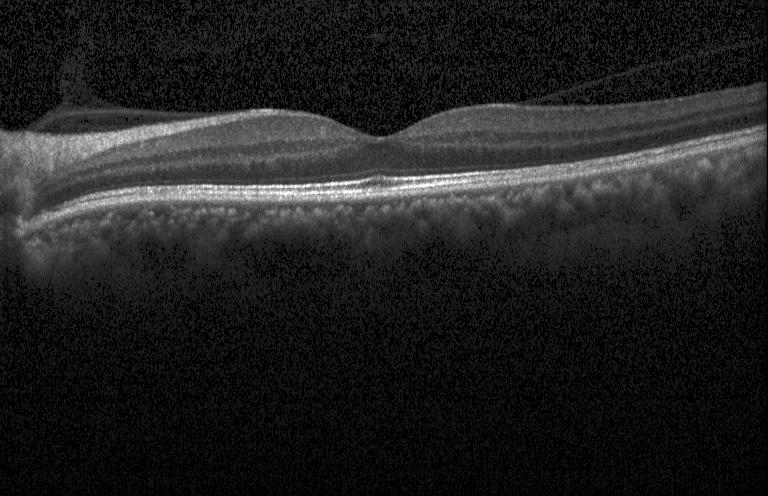 Spectral-domain OCT · Heidelberg Spectralis OCT system · OCT B-scan · centered on the fovea.
This B-scan demonstrates no evidence of choroidal neovascularization, diabetic macular edema, or drusen.